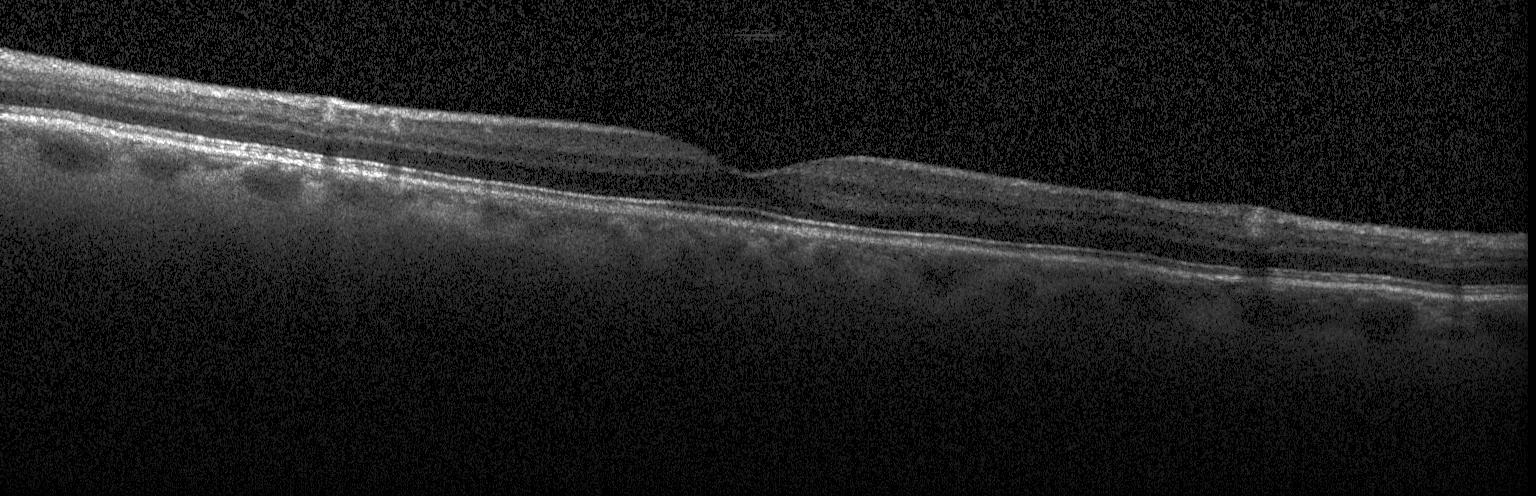
Retinal OCT cross-section
Finding: no evidence of CNV, DME, or drusen.